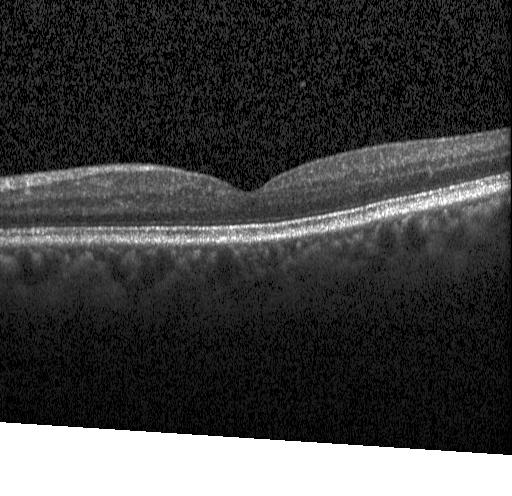
Finding: no choroidal neovascularization, diabetic macular edema, or drusen.